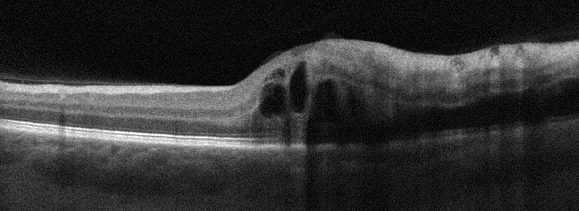
OS · retinal OCT B-scan · Optovue Avanti RTVue XR.
Dx: retinal vein occlusion.